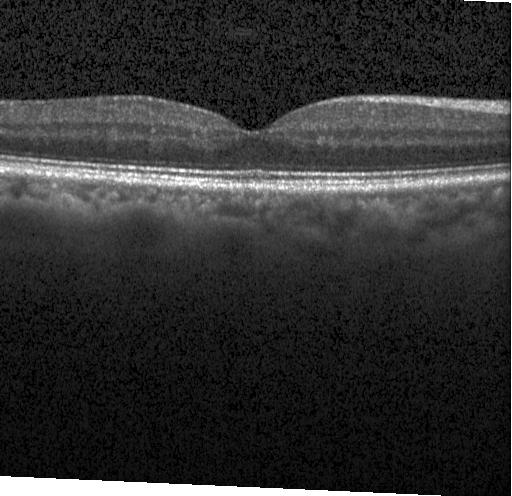 Optical coherence tomography B-scan — Diagnosis: no choroidal neovascularization, diabetic macular edema, or drusen.